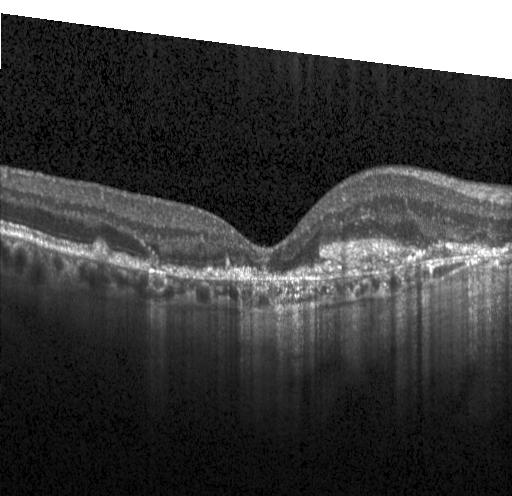
Dx: choroidal neovascularization.